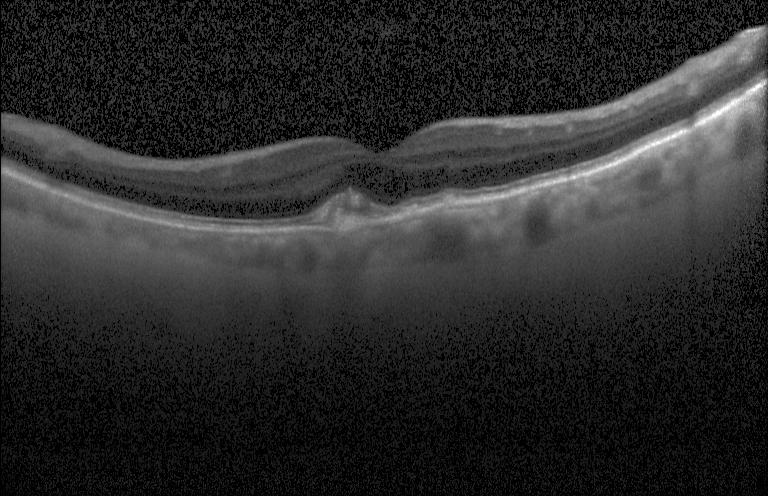

OCT finding: choroidal neovascularization (CNV).